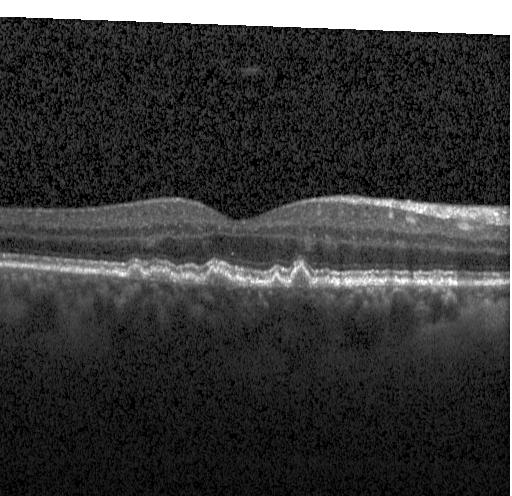

Dx: drusen.